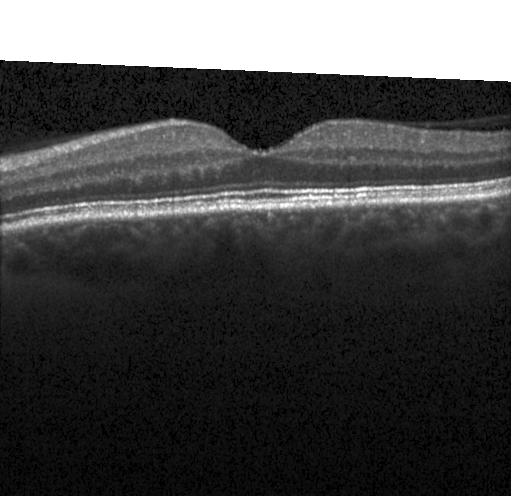

OCT finding: no evidence of choroidal neovascularization, diabetic macular edema, or drusen.